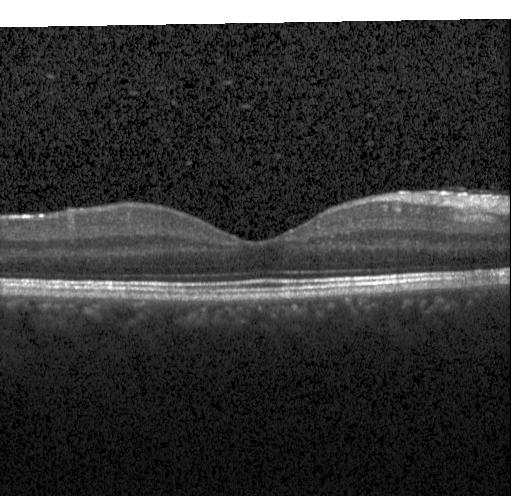

Dx: neither choroidal neovascularization, diabetic macular edema, nor drusen.